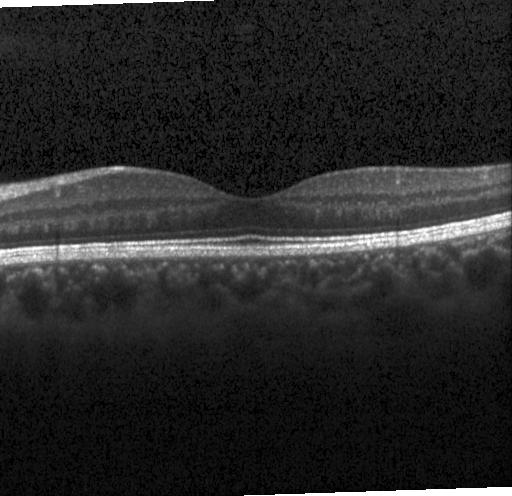
Impression: no evidence of CNV, DME, or drusen.